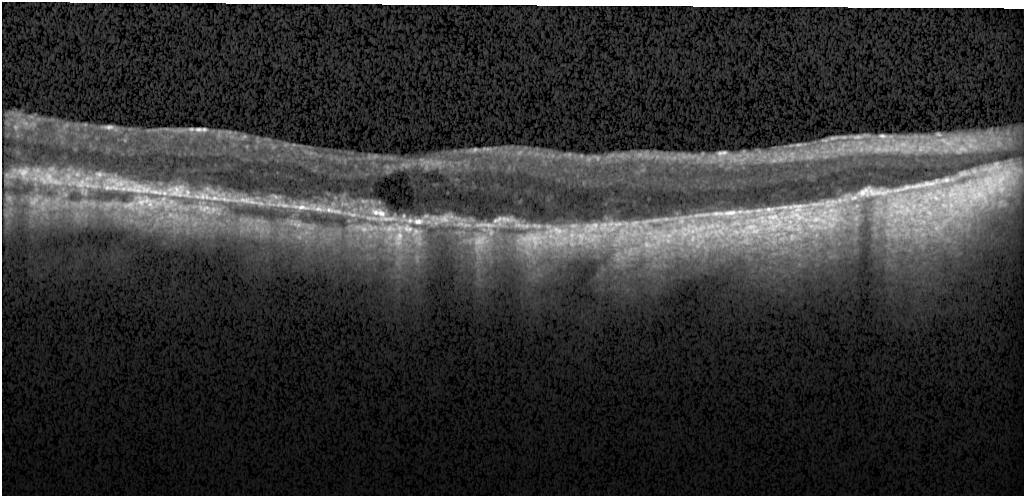
Macular OCT: CNV.